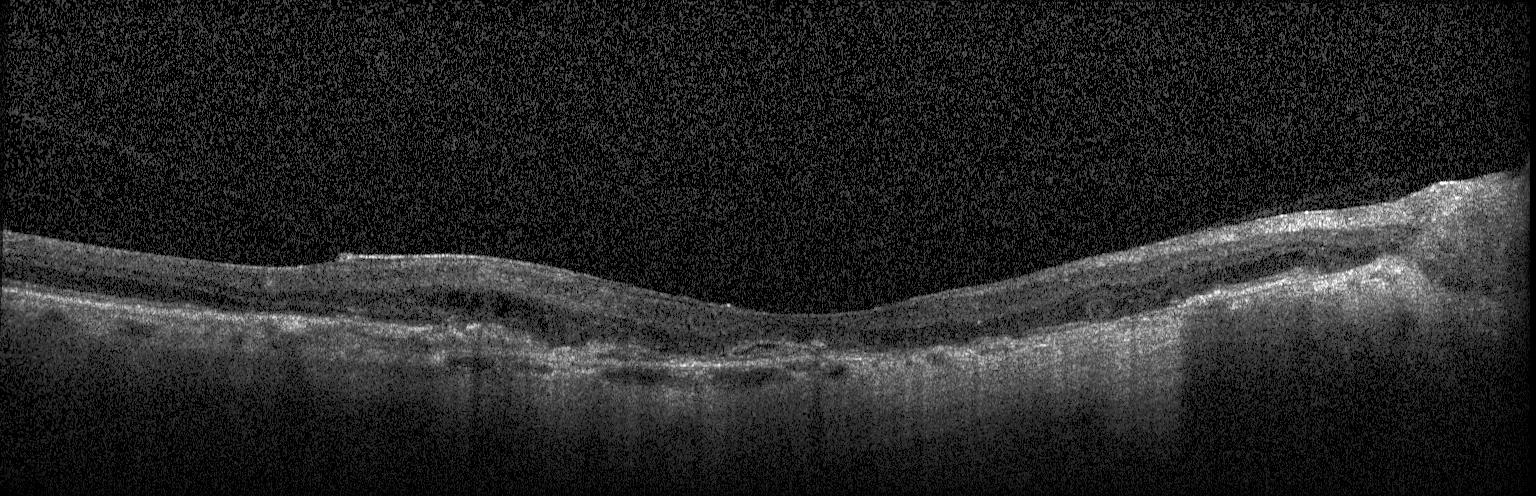
OCT line scan — This B-scan demonstrates a choroidal neovascular membrane.